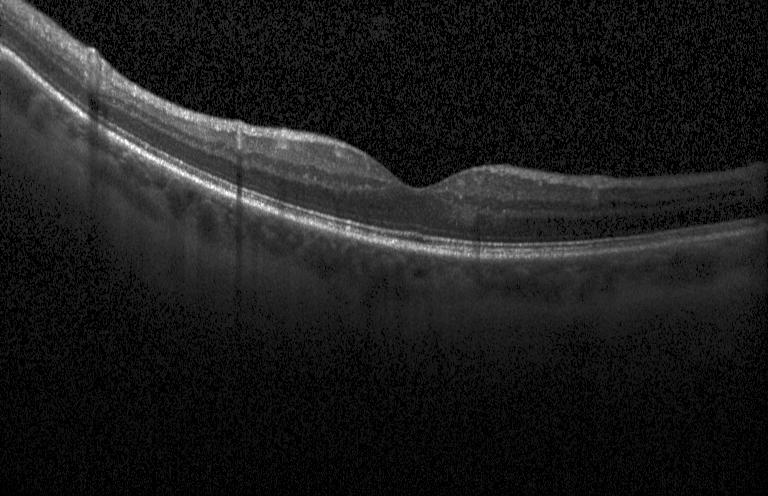

Spectral-domain OCT. Optical coherence tomography scan.
Impression: no evidence of CNV, DME, or drusen.